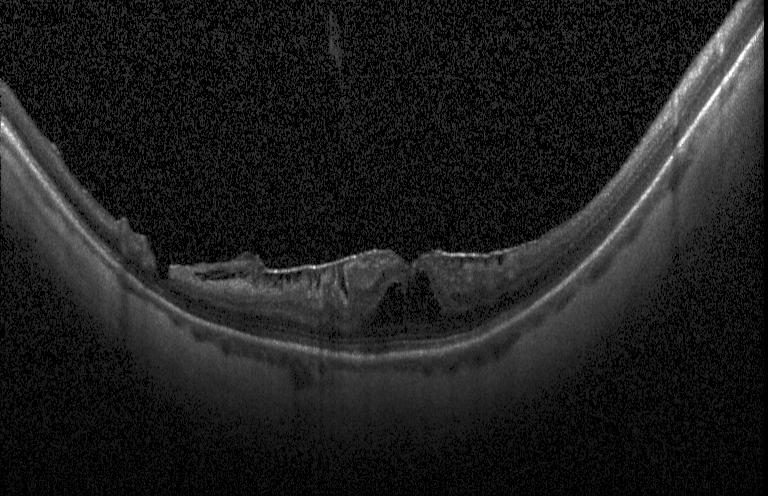 This B-scan demonstrates diabetic macular edema.